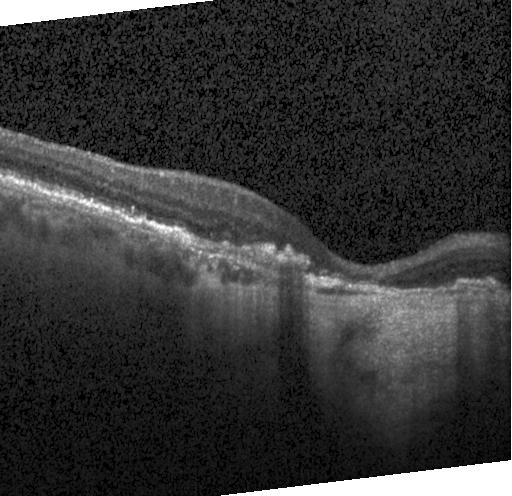
Retinal OCT B-scan. Diagnosis: CNV.